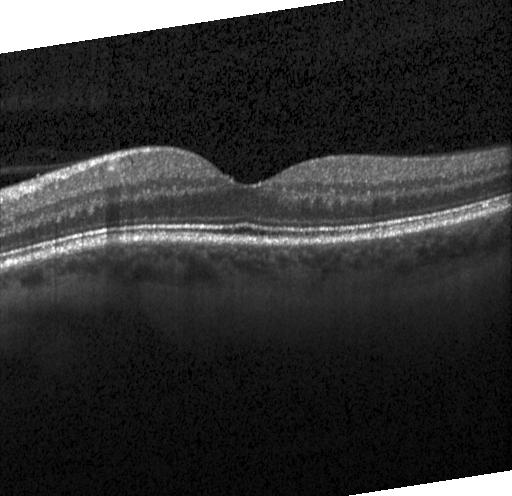
OCT B-scan — OCT finding: no choroidal neovascularization, no diabetic macular edema, and no drusen.